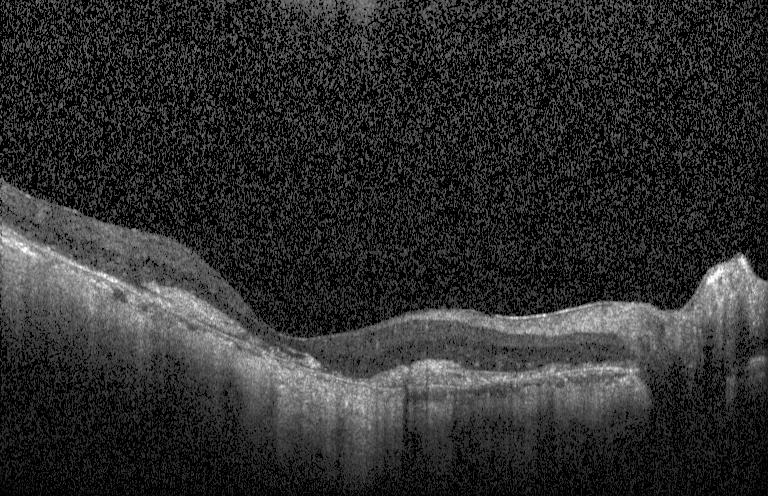
Fovea-centered. SD-OCT. OCT B-scan — Macular OCT: a choroidal neovascular membrane.